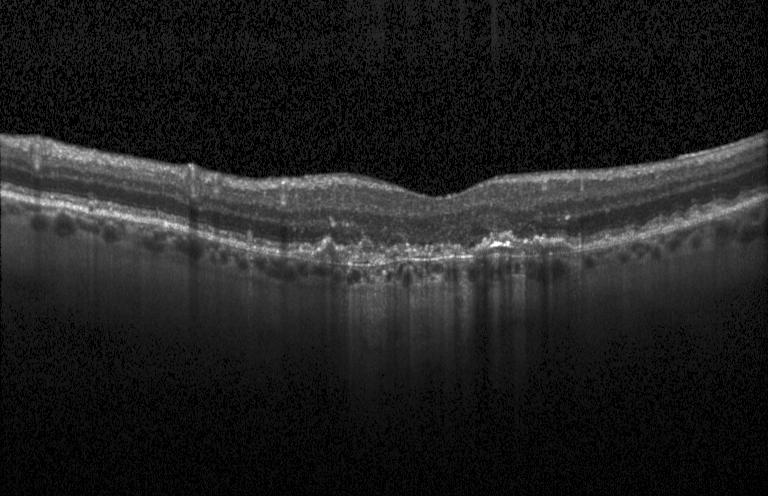
OCT line scan. OCT finding: CNV.